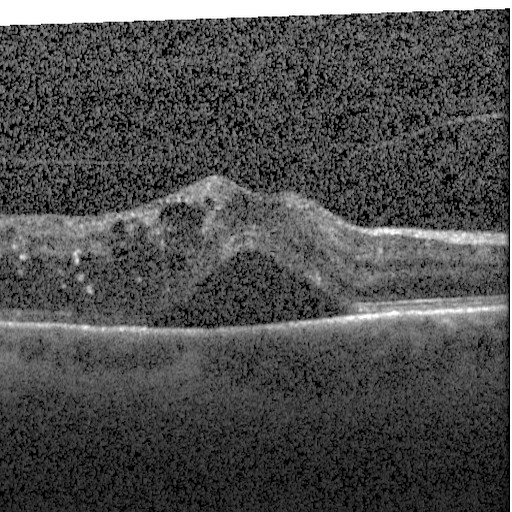 DME.